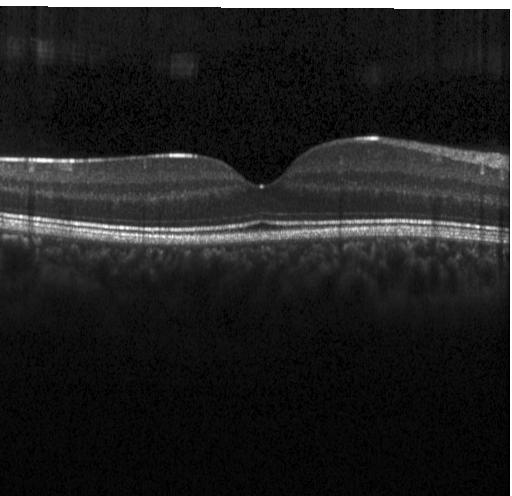
OCT B-scan, acquired on a Heidelberg Spectralis, SD-OCT, through the macula
Diagnosis: no CNV, no DME, and no drusen.